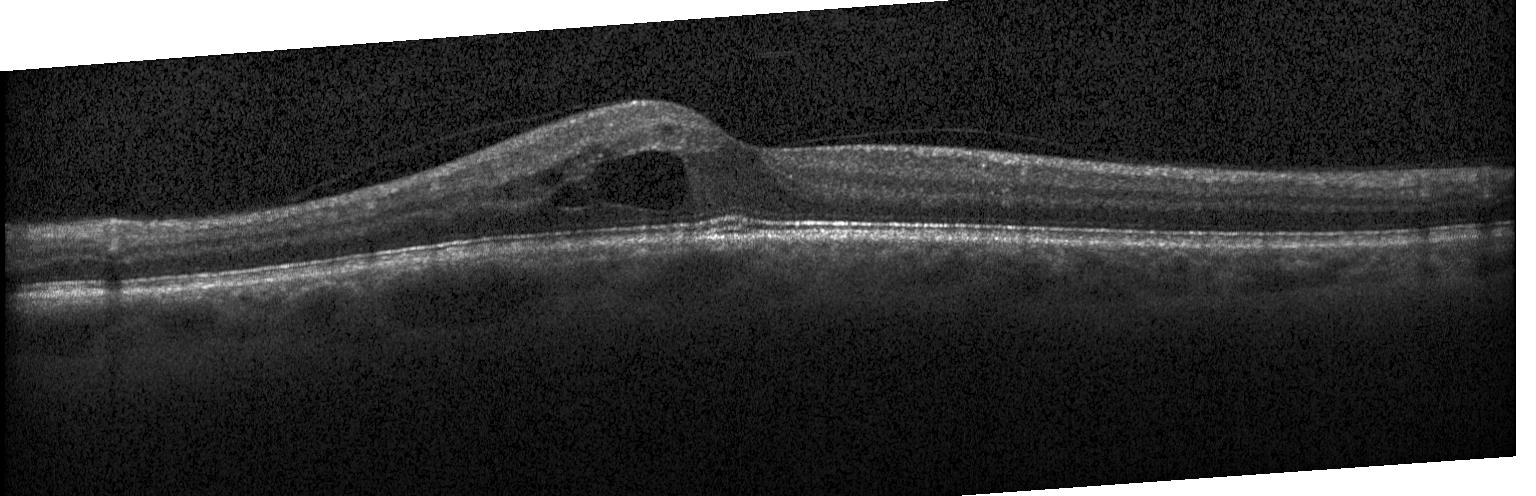
OCT B-scan
Finding: diabetic macular edema.